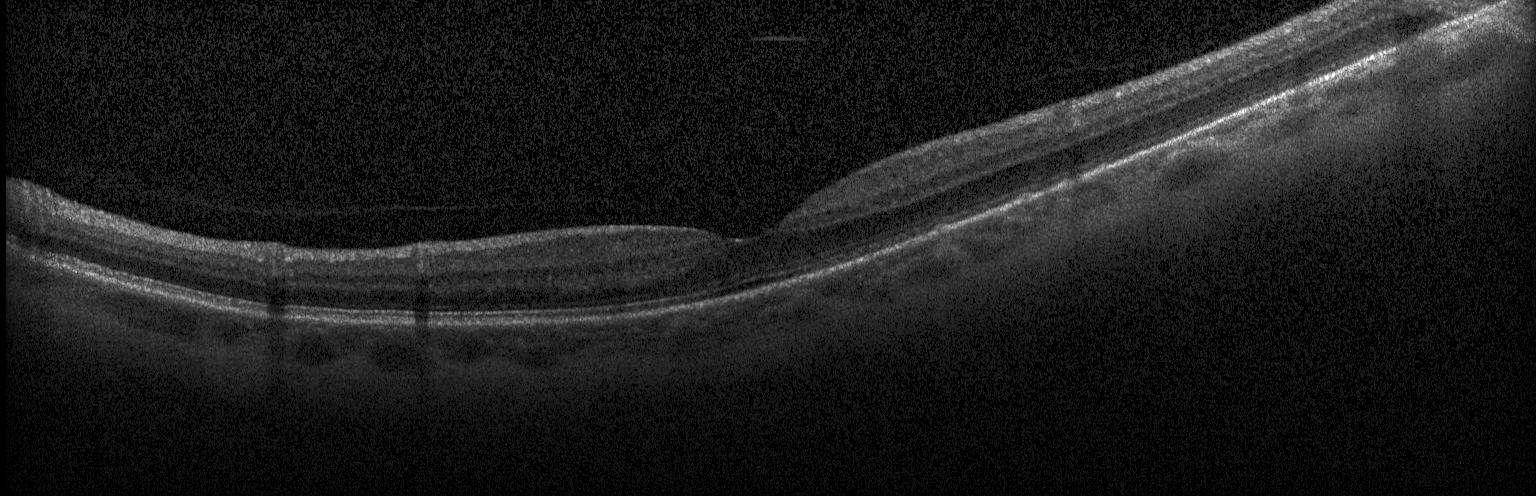
OCT B-scan. Spectral-domain optical coherence tomography. Heidelberg Spectralis — Assessment: no choroidal neovascularization, no diabetic macular edema, and no drusen.